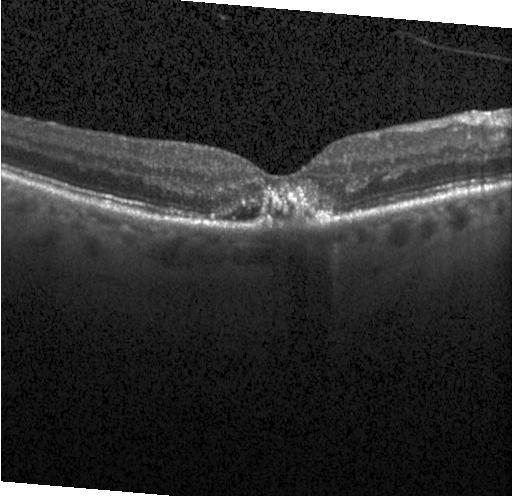 OCT scan showing CNV.